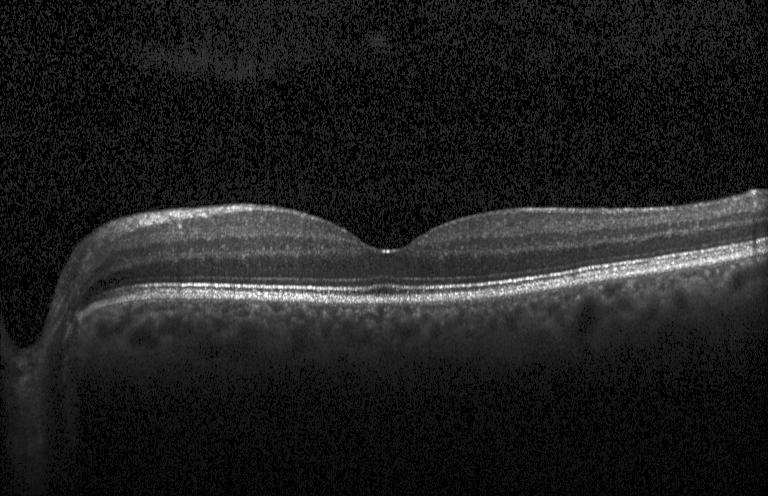
Fovea-centered · optical coherence tomography B-scan · spectral-domain OCT.
This B-scan demonstrates neither choroidal neovascularization, diabetic macular edema, nor drusen.